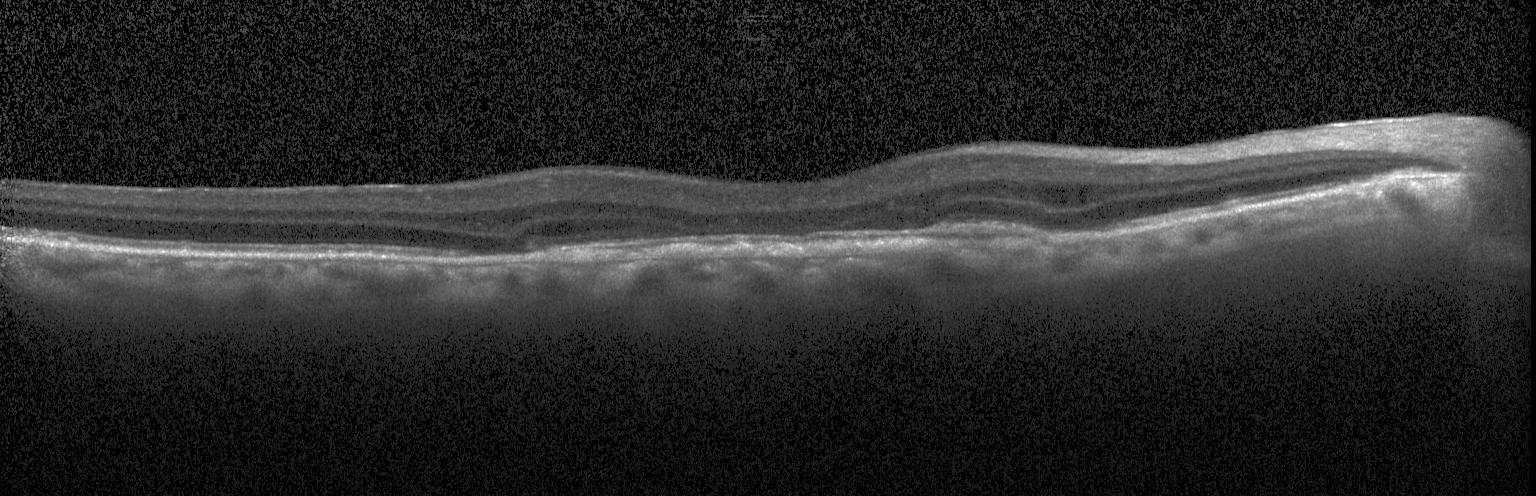
Horizontal scan through the fovea; optical coherence tomography B-scan — Finding: choroidal neovascularization.